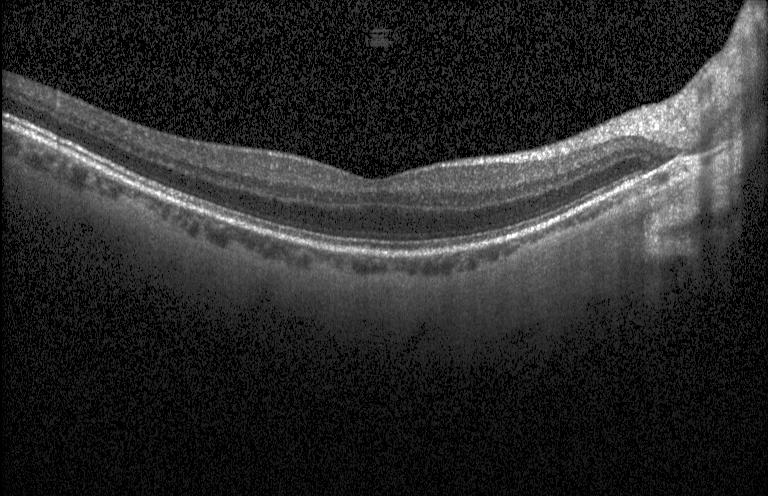
Macular OCT: no choroidal neovascularization, diabetic macular edema, or drusen.